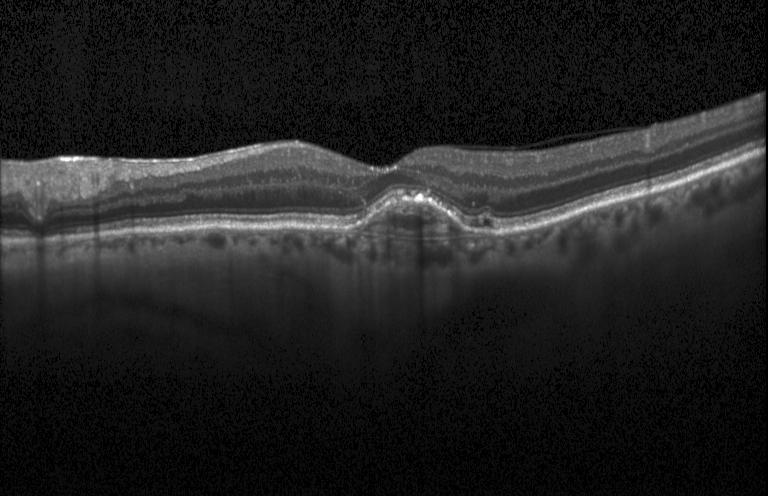 Spectral-domain OCT. Retinal OCT B-scan. Heidelberg Spectralis OCT system
This B-scan demonstrates a choroidal neovascular membrane.